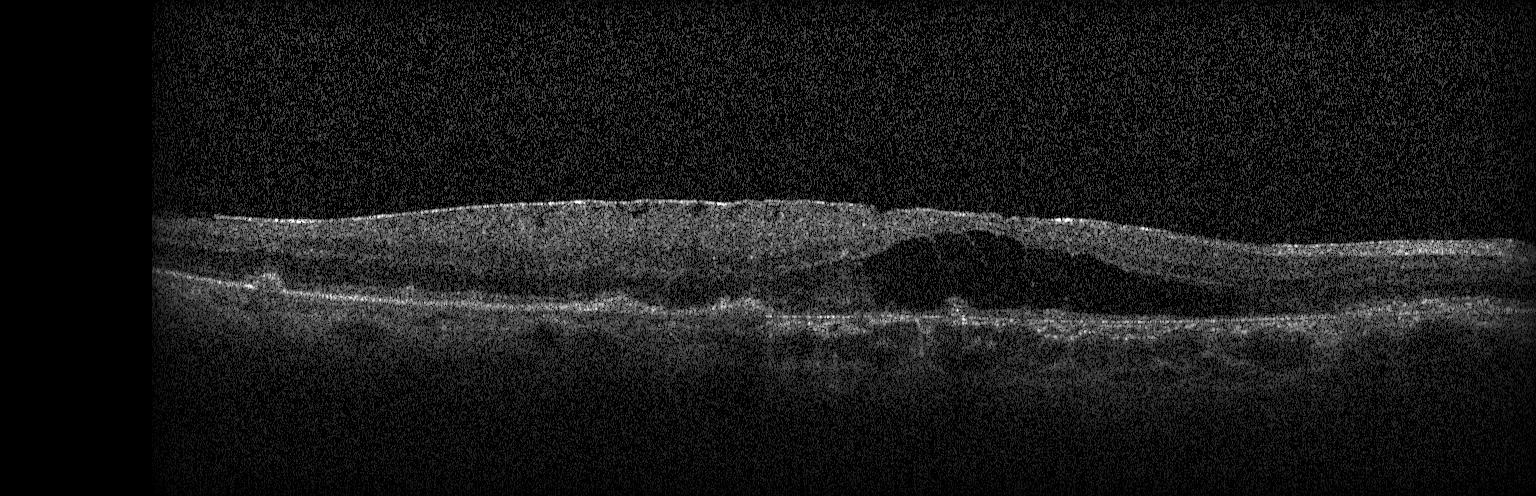

Instrument: Heidelberg Spectralis, optical coherence tomography scan, spectral-domain OCT — Assessment: a choroidal neovascular membrane.